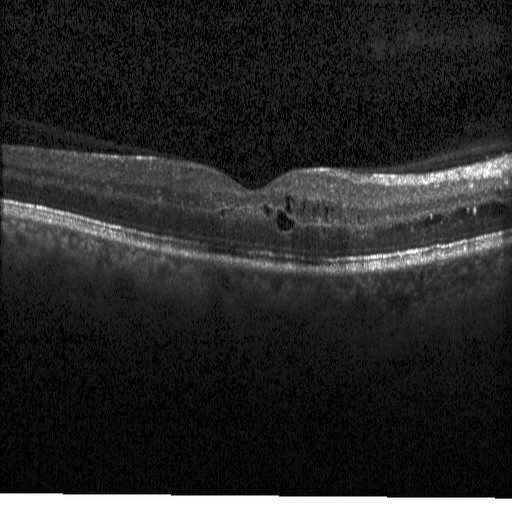 Diabetic macular edema.